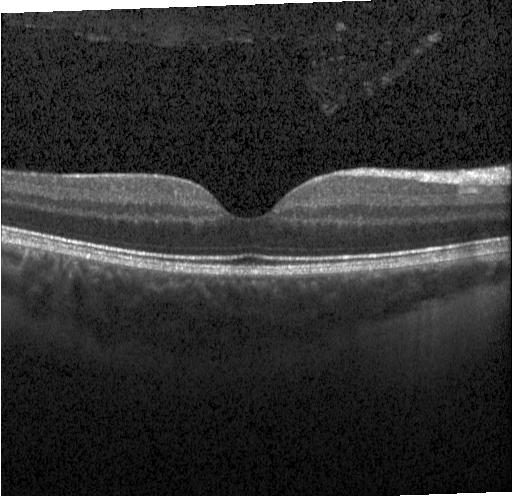
Instrument: Heidelberg Spectralis; spectral-domain optical coherence tomography; OCT line scan — The scan shows neither choroidal neovascularization, diabetic macular edema, nor drusen.